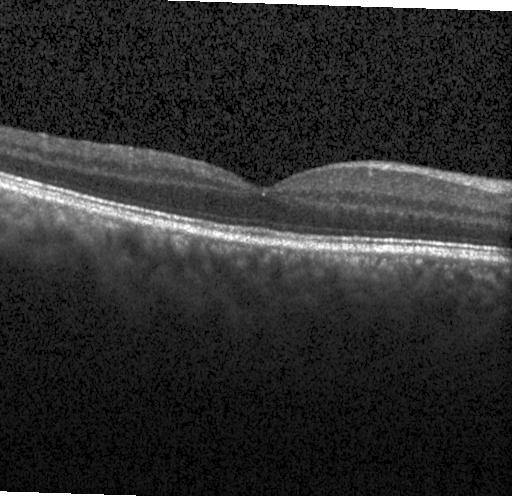 Centered on the fovea · optical coherence tomography scan. This B-scan demonstrates no choroidal neovascularization, no diabetic macular edema, and no drusen.